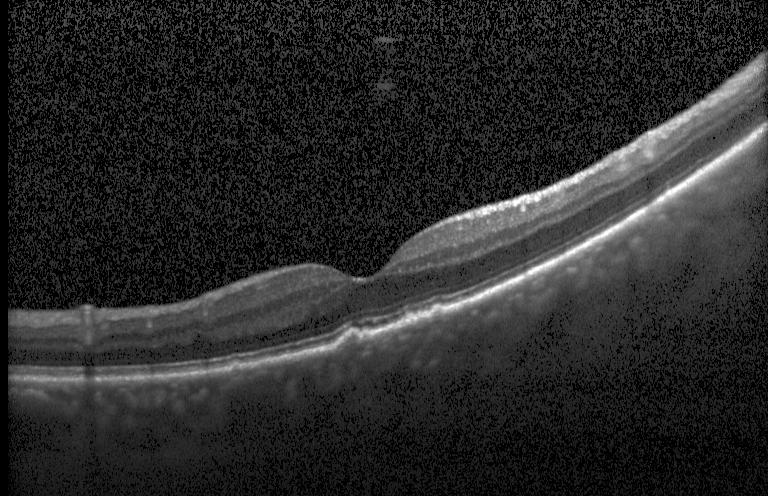 OCT B-scan. Acquired on a Heidelberg Spectralis. SD-OCT — Impression: multiple drusen.